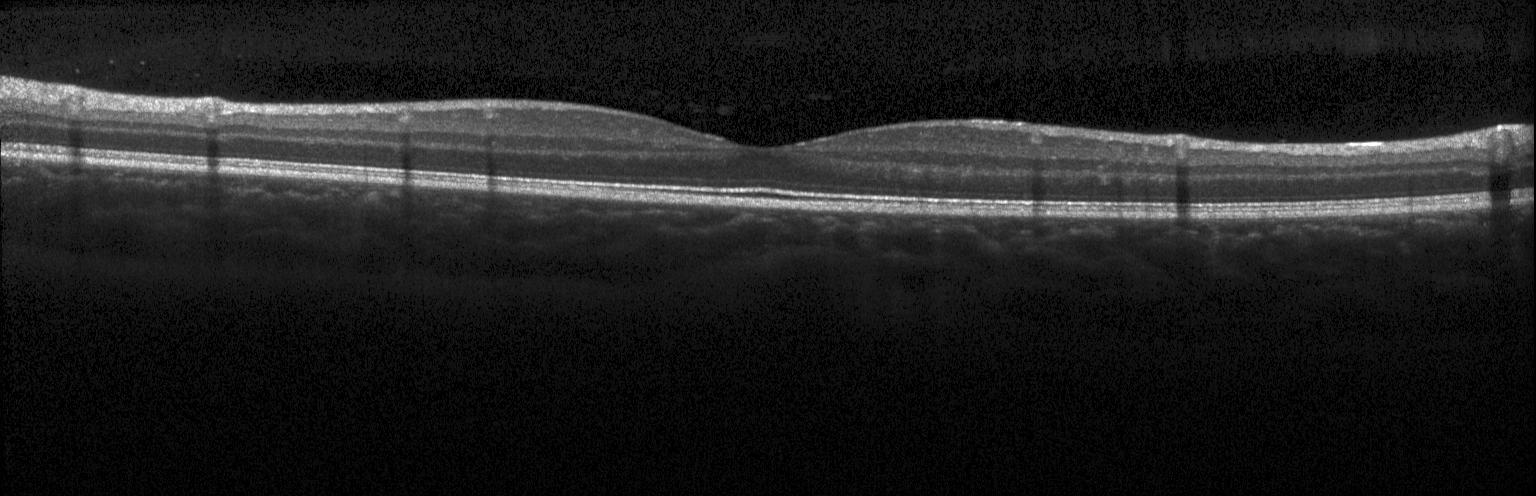
Macular scan; Heidelberg Spectralis OCT system; OCT line scan. Dx: no evidence of CNV, DME, or drusen.